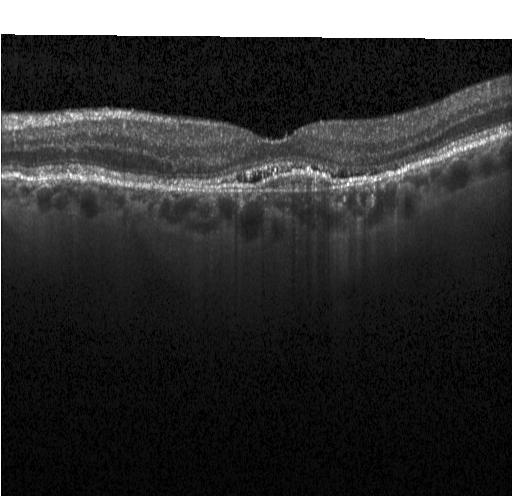

Macular OCT: a choroidal neovascular membrane.